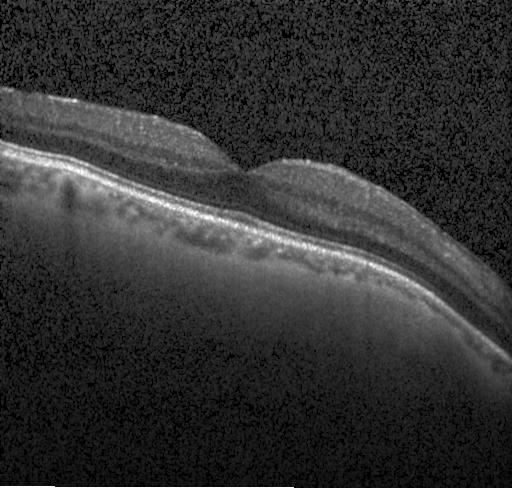 OCT finding: neither choroidal neovascularization, diabetic macular edema, nor drusen.